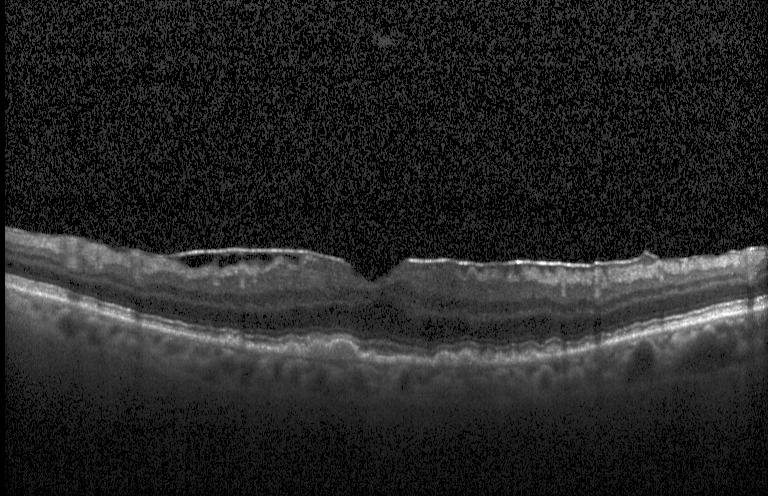
Optical coherence tomography scan — Impression: drusen.